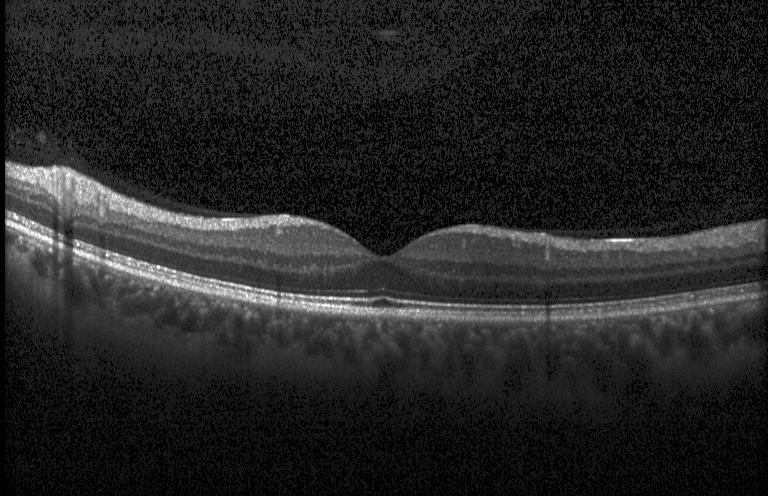 The scan shows no choroidal neovascularization, no diabetic macular edema, and no drusen.